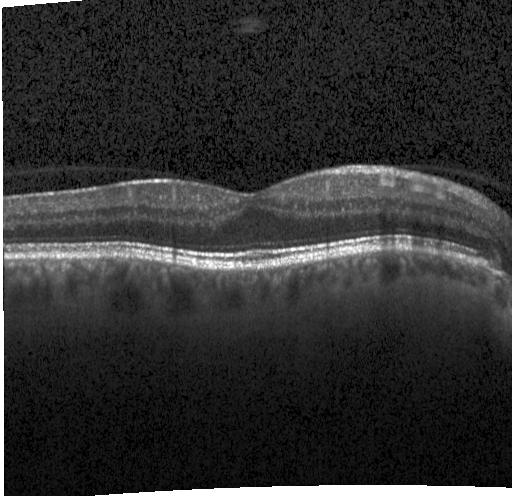

Retinal OCT B-scan. Diagnosis: no choroidal neovascularization, no diabetic macular edema, and no drusen.